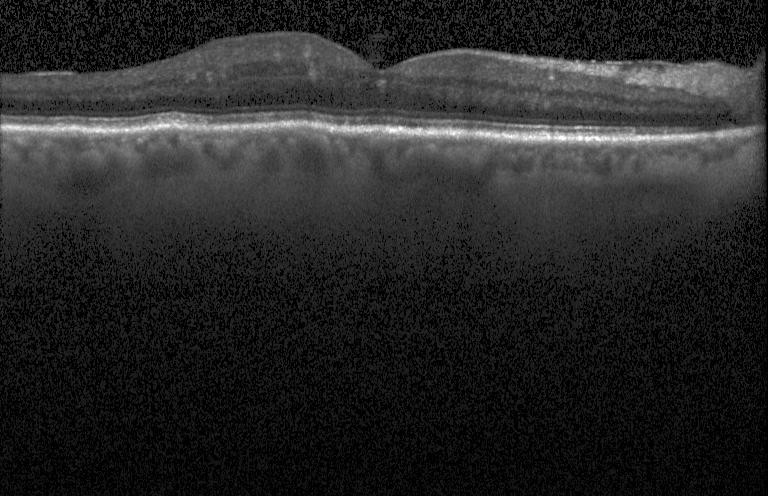
Diagnosis: neither choroidal neovascularization, diabetic macular edema, nor drusen.